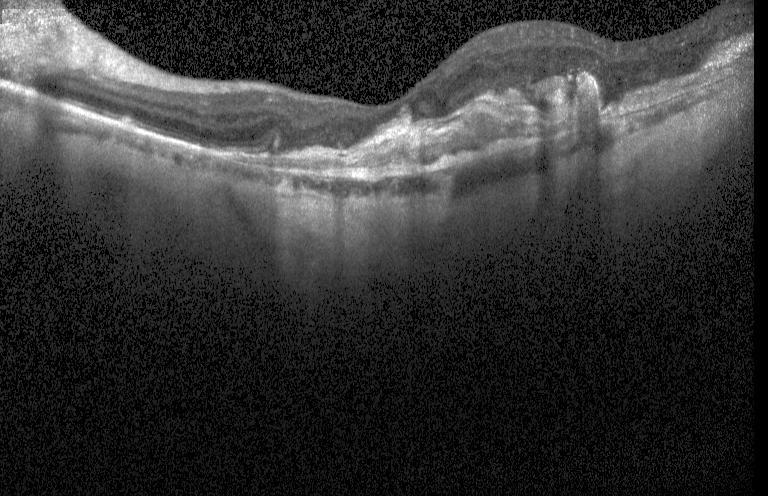 SD-OCT; retinal OCT cross-section — A choroidal neovascular membrane.